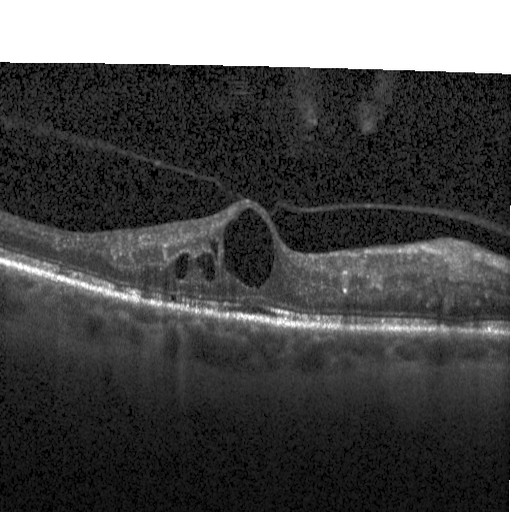
Dx: diabetic macular edema.